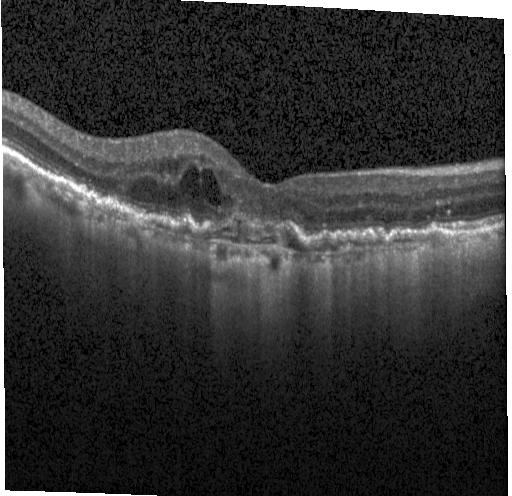
Horizontal scan through the fovea, instrument: Heidelberg Spectralis, spectral-domain optical coherence tomography, retinal OCT B-scan. Assessment: CNV.